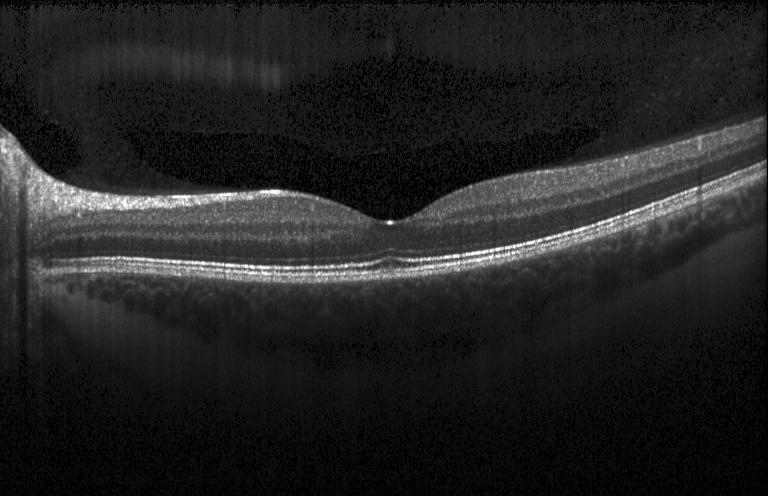 Spectral-domain optical coherence tomography; Heidelberg Spectralis OCT system; centered on the fovea; OCT B-scan — The scan shows no evidence of CNV, DME, or drusen.